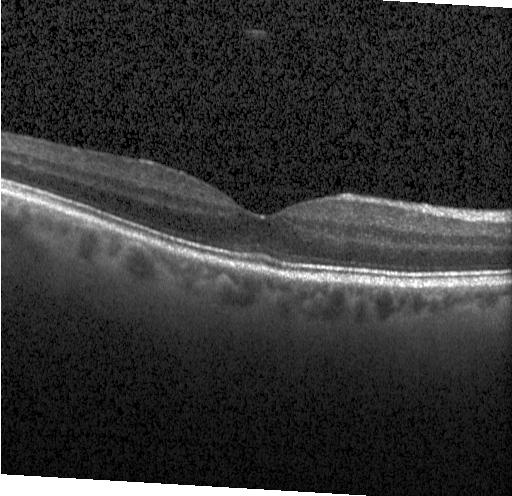

Finding: neither CNV, DME, nor drusen.